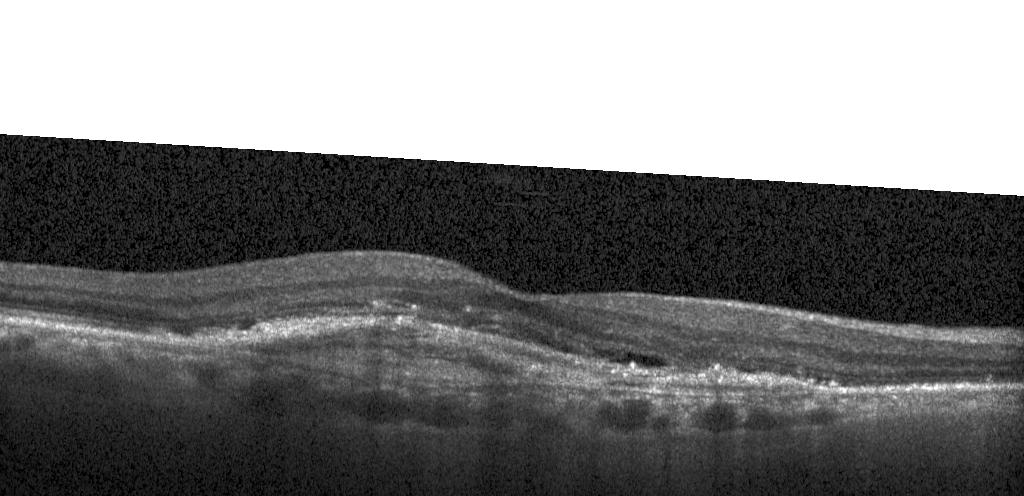
Instrument: Heidelberg Spectralis, OCT line scan, SD-OCT. This B-scan demonstrates a choroidal neovascular membrane.